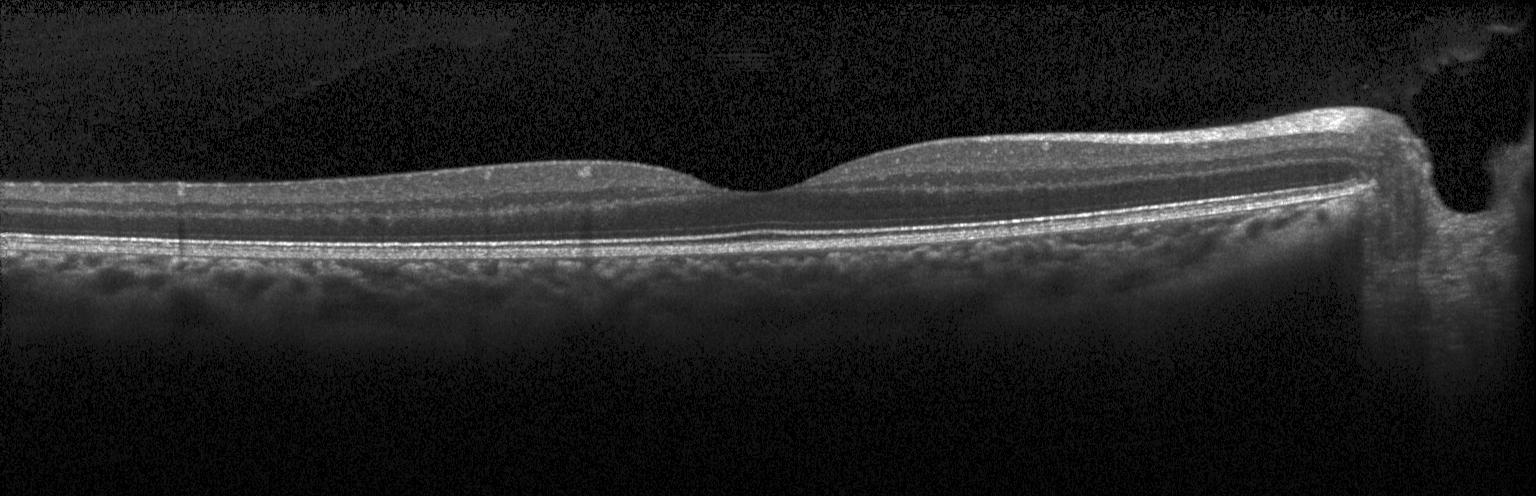 Impression: no evidence of choroidal neovascularization, diabetic macular edema, or drusen.